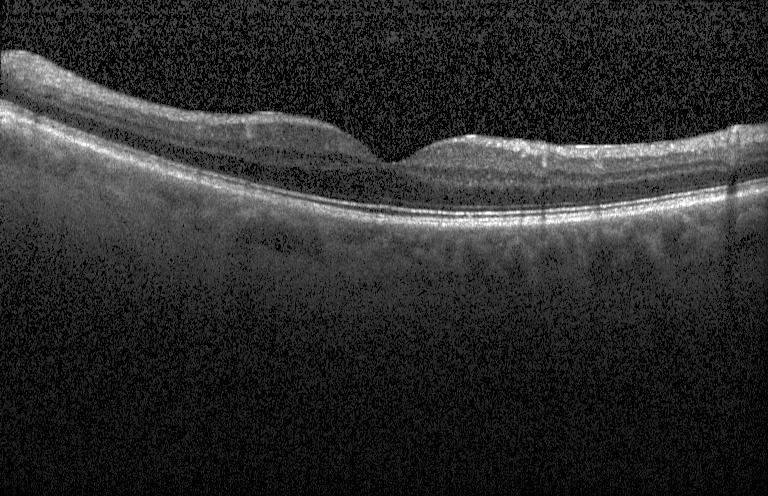

Dx: no choroidal neovascularization, diabetic macular edema, or drusen.